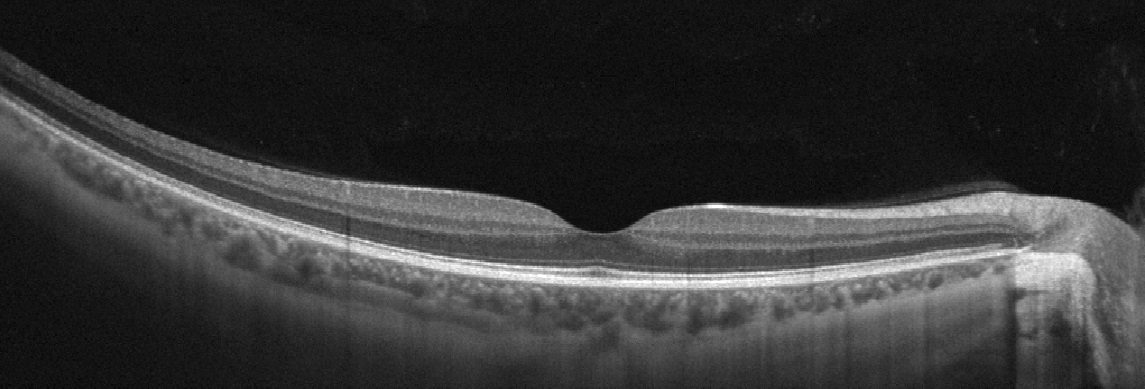 Retinal OCT B-scan · through the macula. Impression: no evidence of AMD, DME, ERM, RAO, RVO, or VID.